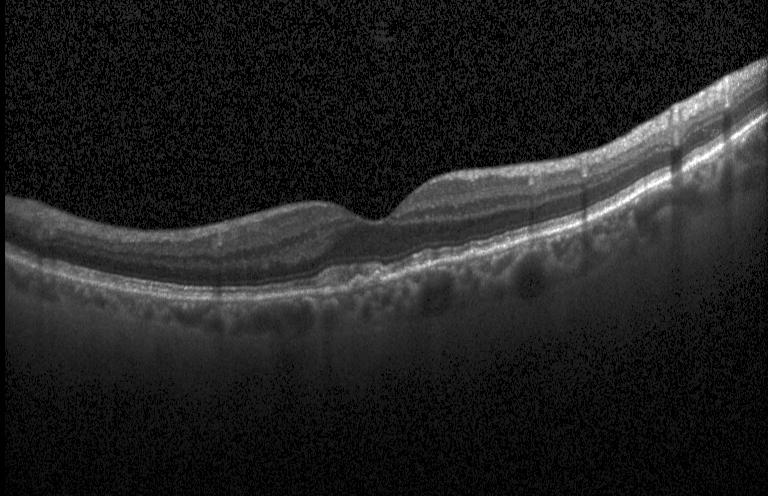

This B-scan demonstrates sub-RPE drusenoid deposits.